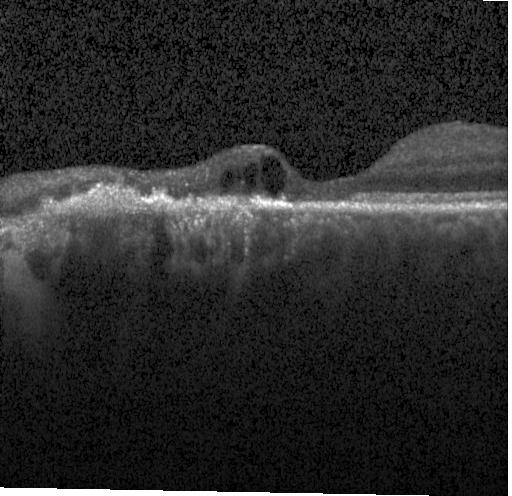 Macular OCT demonstrating a choroidal neovascular membrane.